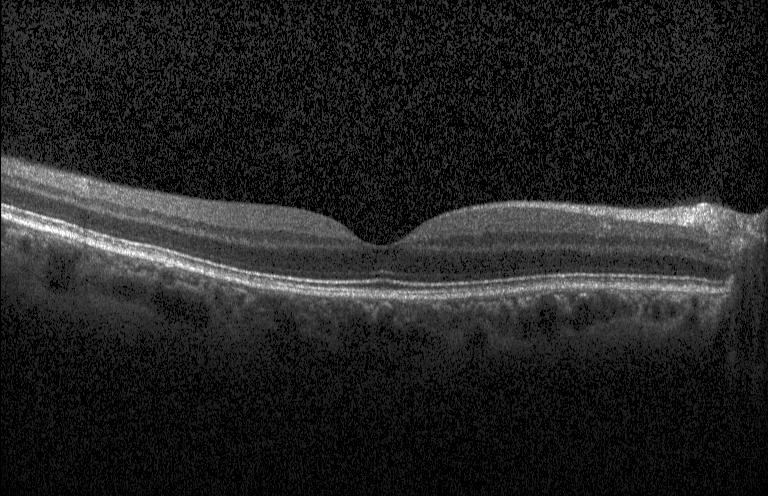
Diagnosis: no CNV, DME, or drusen.